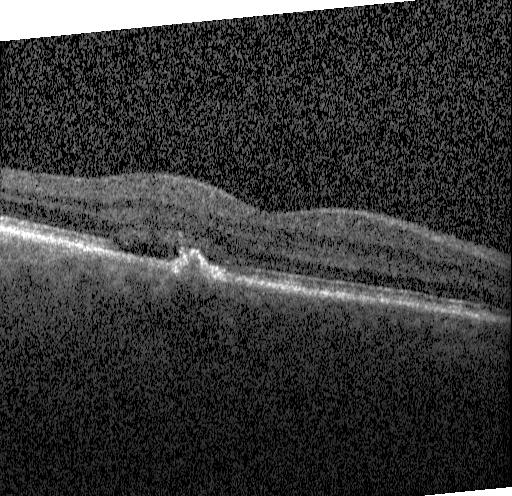

The scan shows choroidal neovascularization.